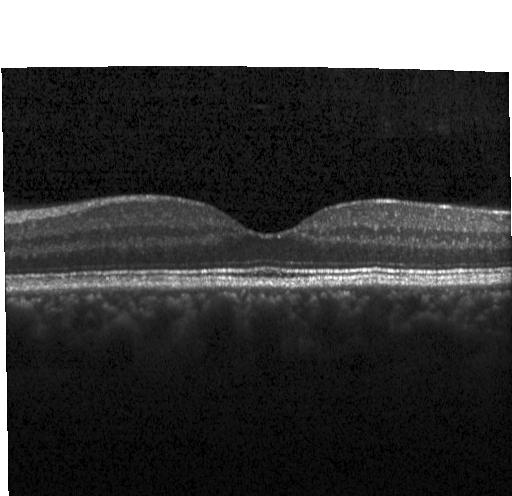
Acquired on a Heidelberg Spectralis; spectral-domain OCT; optical coherence tomography B-scan
OCT finding: no choroidal neovascularization, diabetic macular edema, or drusen.